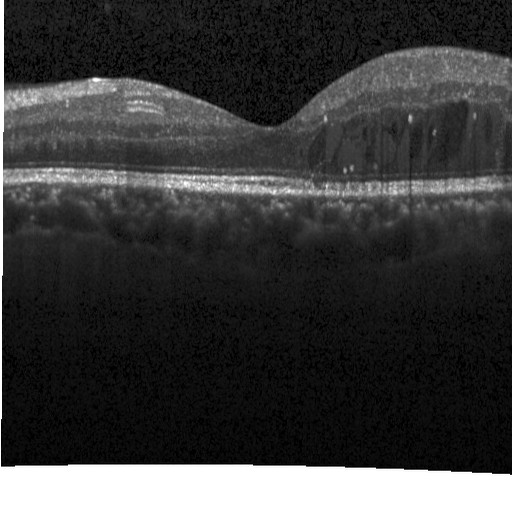

Spectral-domain OCT B-scan: diabetic macular edema (DME).